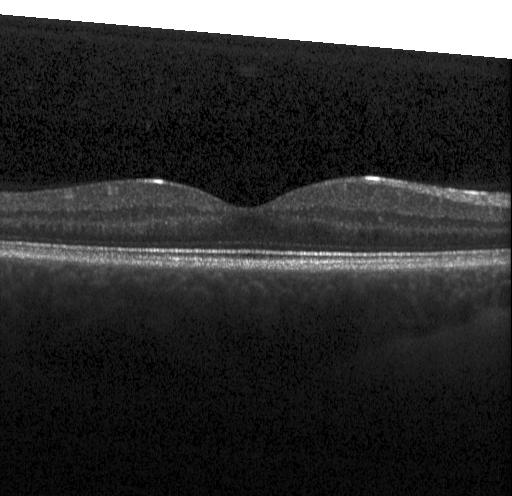 Optical coherence tomography B-scan. The scan shows no CNV, DME, or drusen.